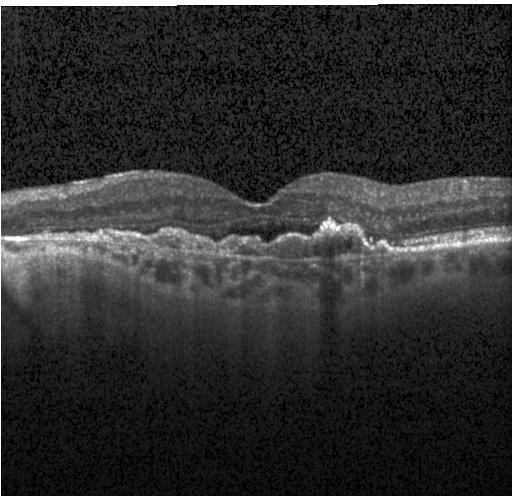 SD-OCT · centered on the fovea · optical coherence tomography scan
Assessment: a choroidal neovascular membrane.